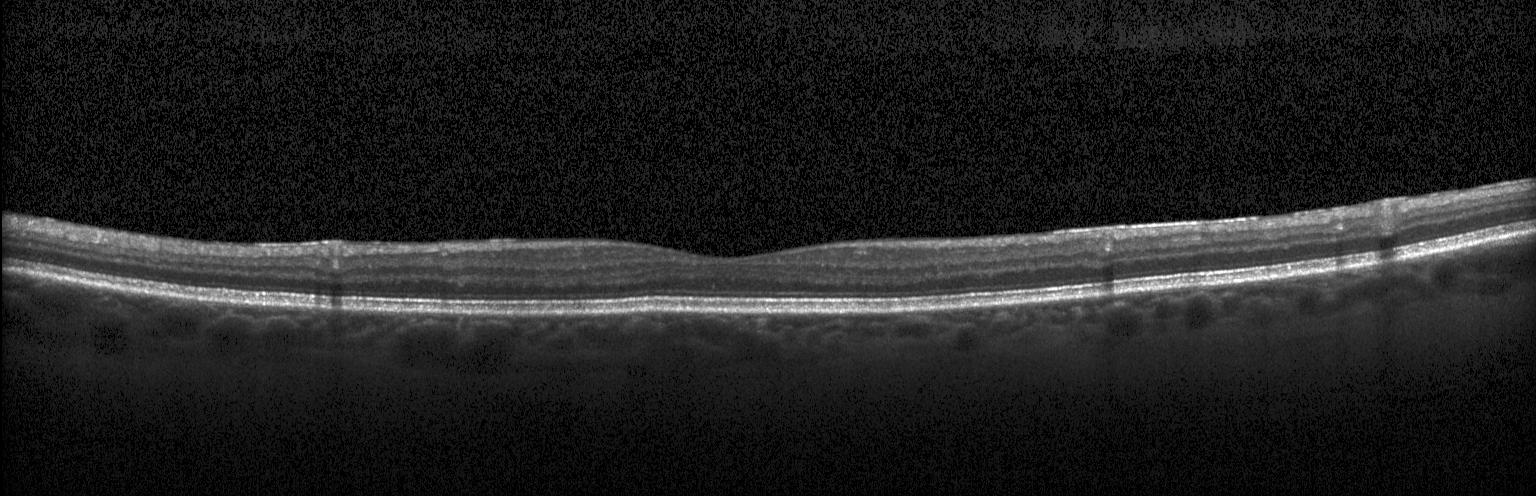

Retinal OCT B-scan — Diagnosis: neither choroidal neovascularization, diabetic macular edema, nor drusen.